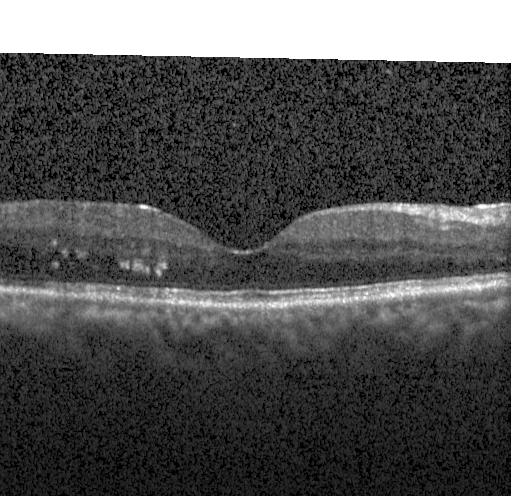 Impression: DME.